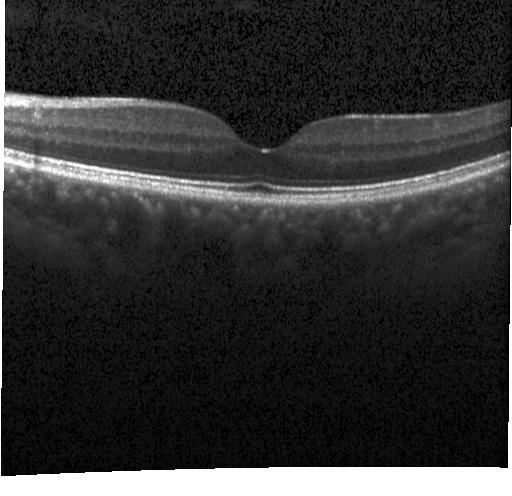
Assessment: no evidence of CNV, DME, or drusen.